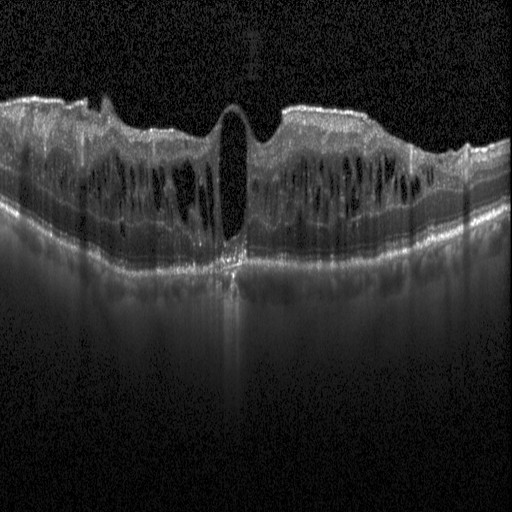
OCT line scan. Finding: DME.